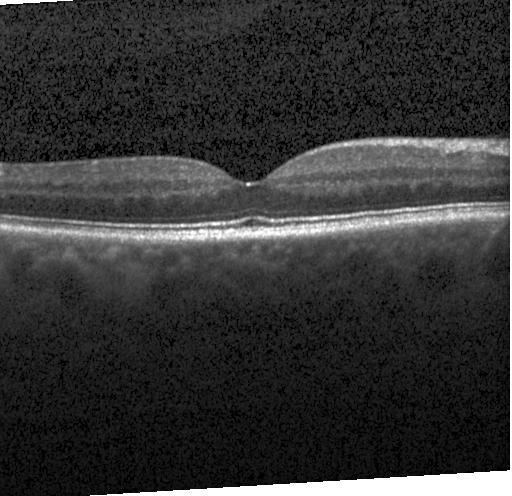
Impression: neither CNV, DME, nor drusen.